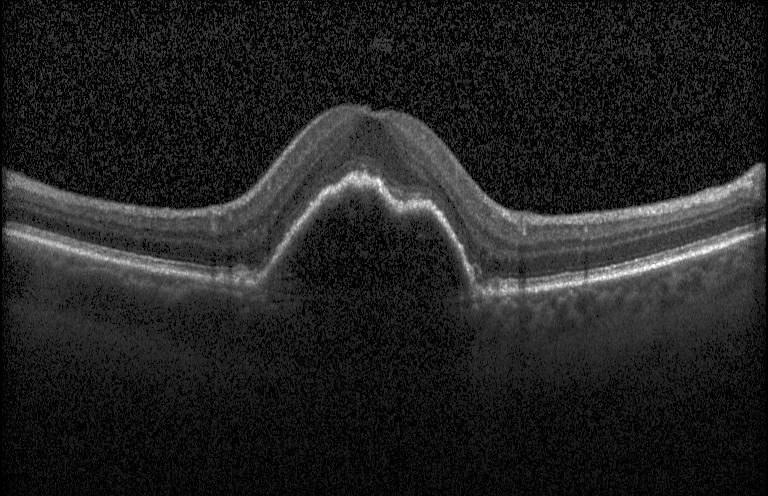

OCT scan showing a choroidal neovascular membrane.